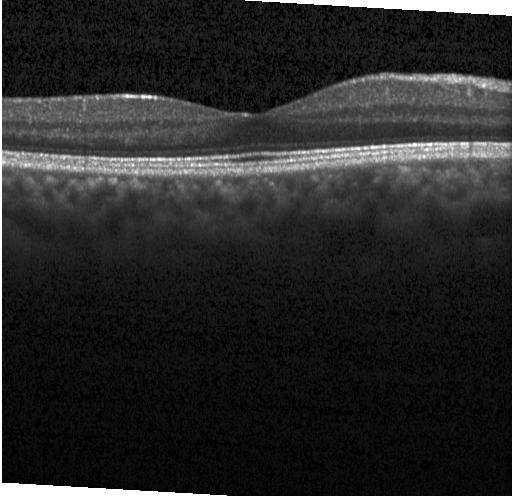

Macular scan · retinal OCT B-scan · spectral-domain OCT. Diagnosis: neither choroidal neovascularization, diabetic macular edema, nor drusen.